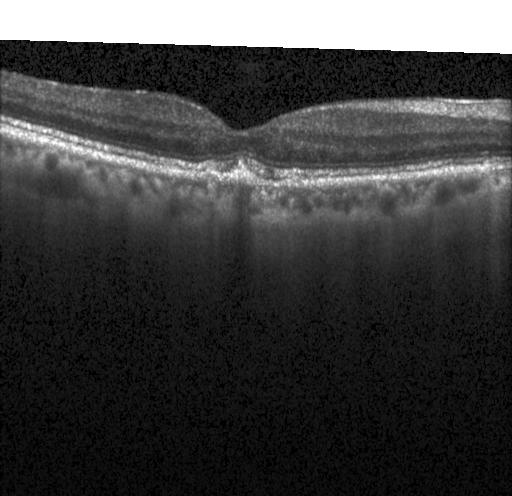
Optical coherence tomography B-scan.
Finding: choroidal neovascularization.